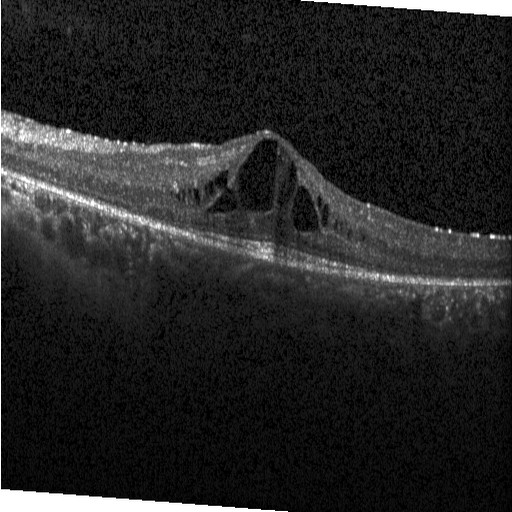

Finding: diabetic macular edema (DME).